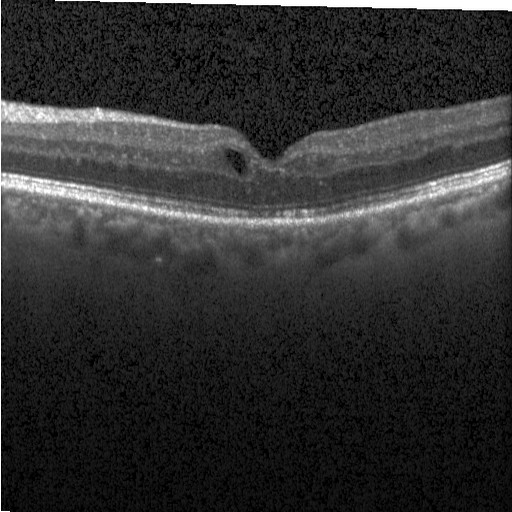 Optical coherence tomography scan. Macular OCT: diabetic macular edema (DME).